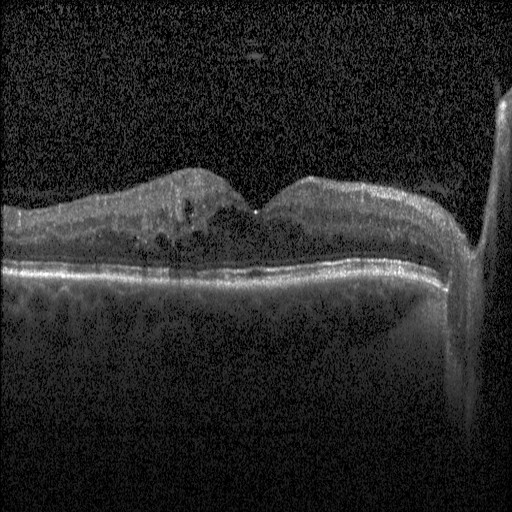 OCT B-scan — The scan shows diabetic macular edema (DME).